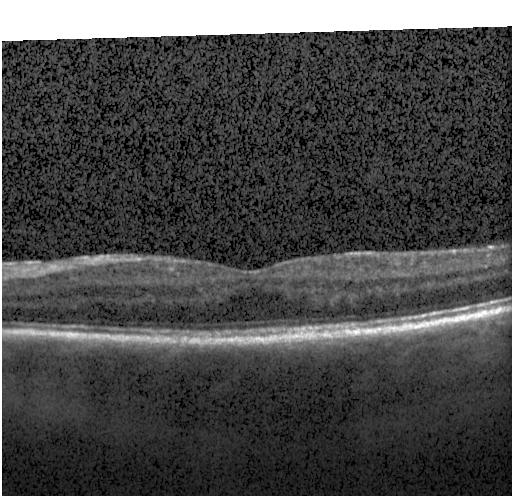

Heidelberg Spectralis, retinal OCT cross-section, spectral-domain optical coherence tomography, centered on the fovea.
Impression: no choroidal neovascularization, no diabetic macular edema, and no drusen.